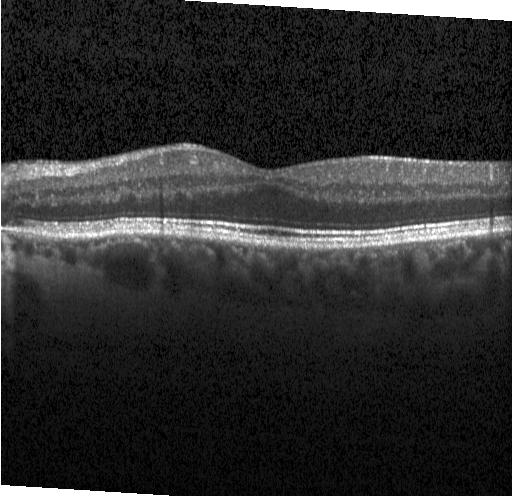
Spectral-domain OCT B-scan: no evidence of choroidal neovascularization, diabetic macular edema, or drusen.